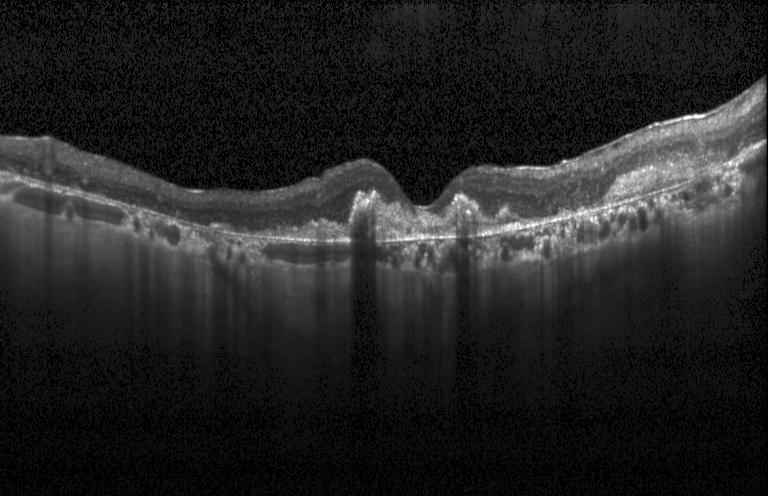 Retinal OCT cross-section. Instrument: Heidelberg Spectralis — Dx: a choroidal neovascular membrane.